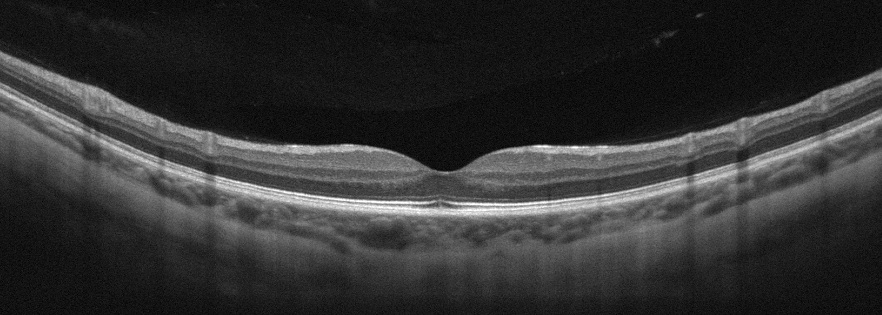
OS; retinal OCT B-scan
Impression: no evidence of AMD, DME, ERM, RAO, RVO, or VID.